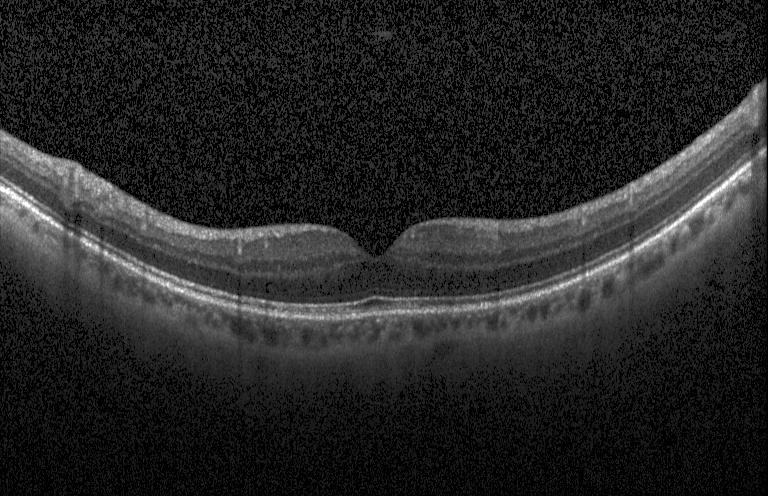

Macular OCT demonstrating no CNV, no DME, and no drusen.